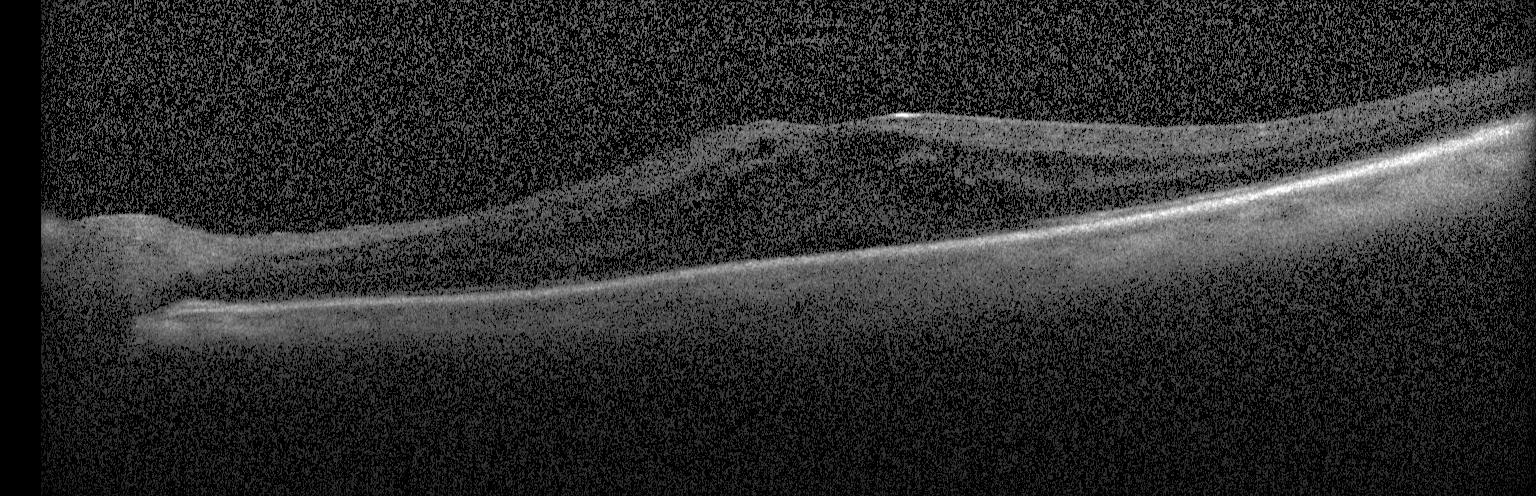 Macular scan · spectral-domain OCT · instrument: Heidelberg Spectralis · OCT B-scan. This B-scan demonstrates DME.